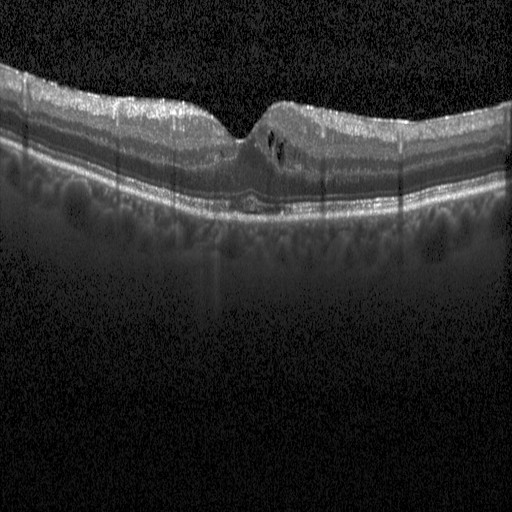
OCT line scan · Heidelberg Spectralis.
Impression: diabetic macular edema (DME).